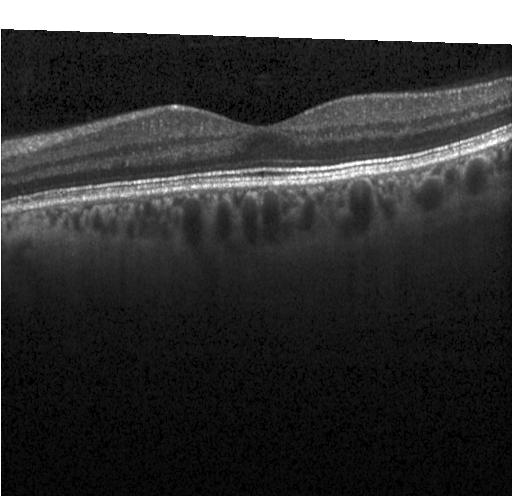

OCT finding: no choroidal neovascularization, no diabetic macular edema, and no drusen.